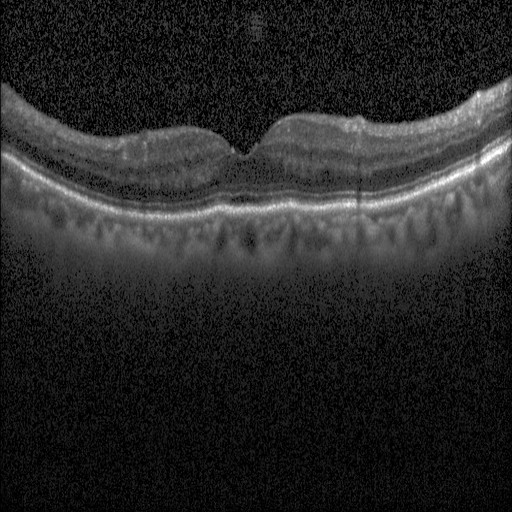
OCT B-scan.
OCT finding: diabetic macular edema.